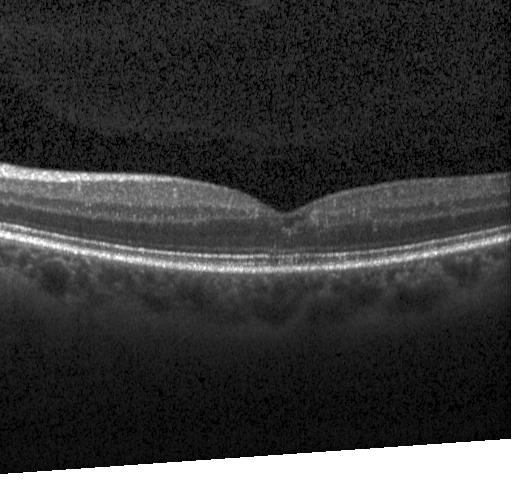

Neither CNV, DME, nor drusen.